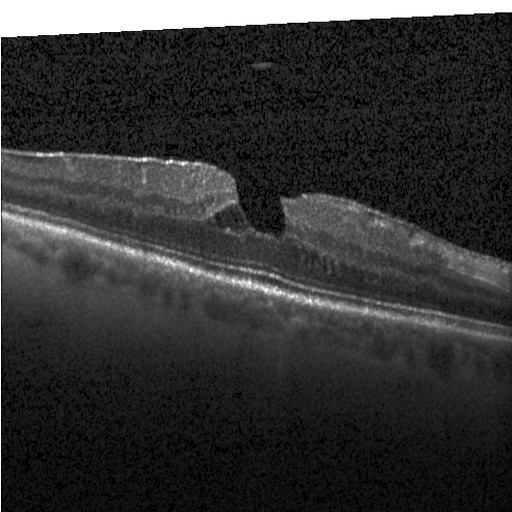
Retinal OCT cross-section, Heidelberg Spectralis OCT system, SD-OCT, through the macula. Finding: DME.